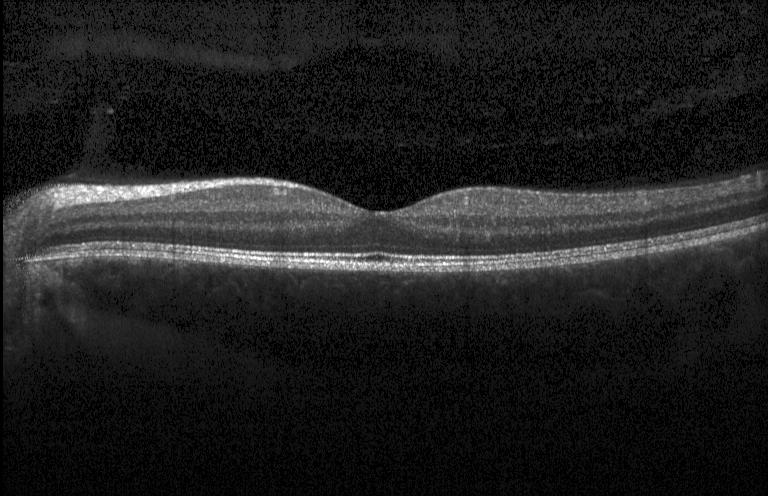

Impression: no evidence of choroidal neovascularization, diabetic macular edema, or drusen.